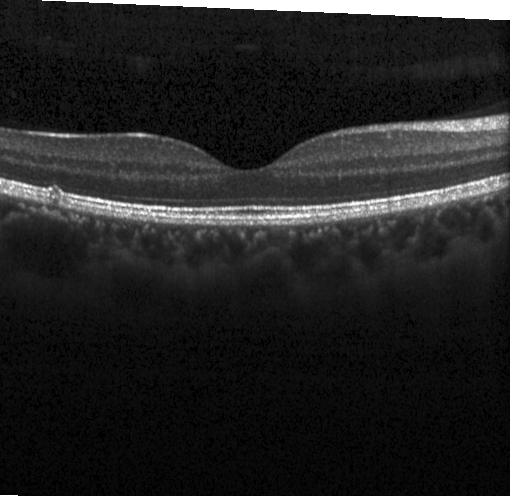

Optical coherence tomography scan.
The scan shows multiple drusen.